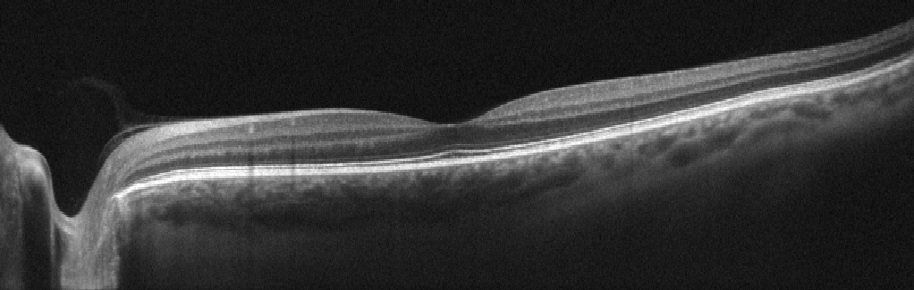 Diagnosis: no evidence of AMD, DME, ERM, RAO, RVO, or VID.